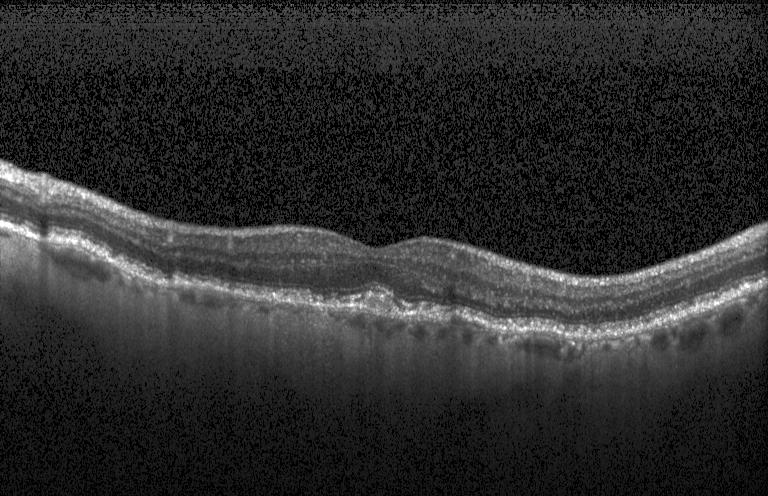 Macular OCT demonstrating multiple drusen.